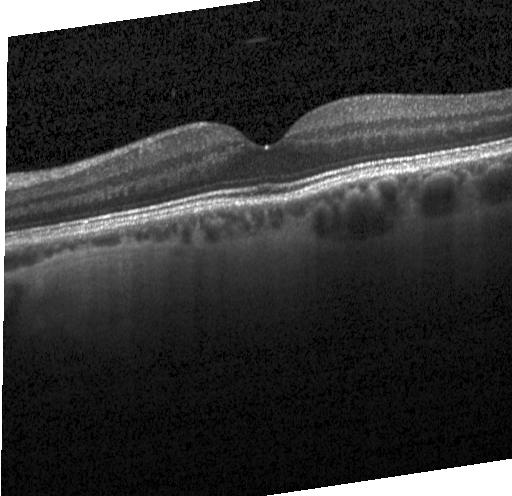
This B-scan demonstrates no evidence of choroidal neovascularization, diabetic macular edema, or drusen.